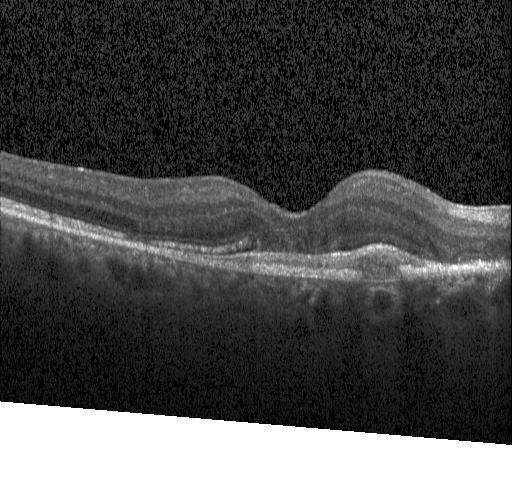 OCT line scan — Macular OCT: choroidal neovascularization.